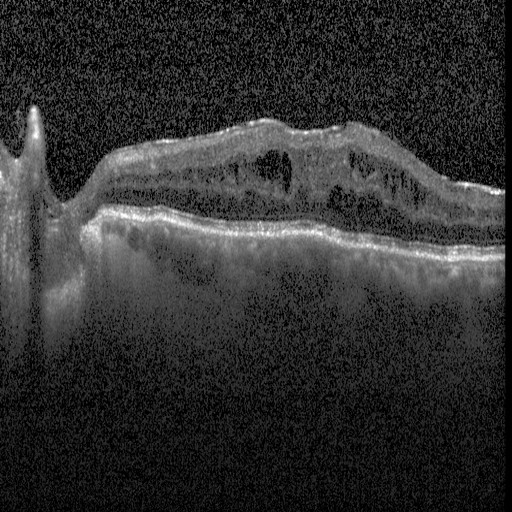
OCT B-scan. The scan shows DME.